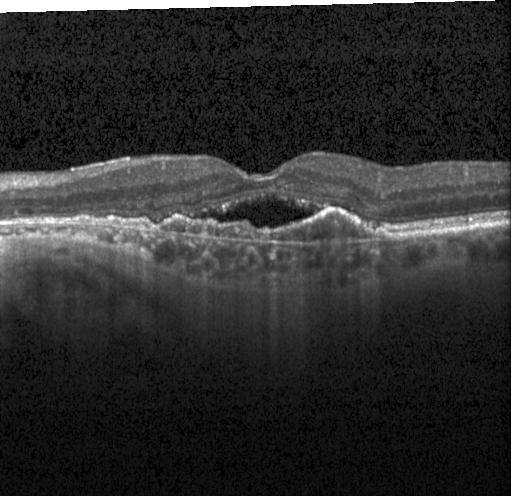
Assessment: choroidal neovascularization (CNV).